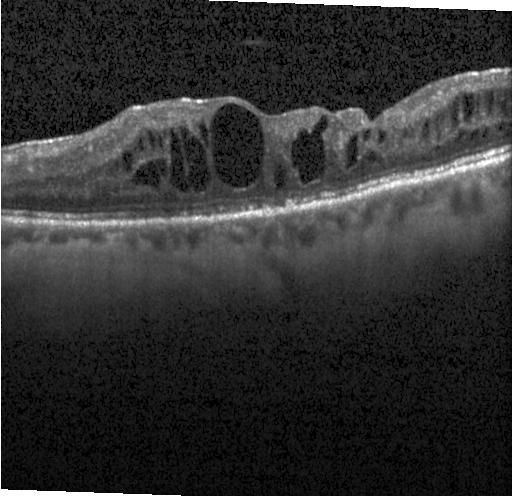 OCT B-scan; Heidelberg Spectralis OCT system; fovea-centered.
The scan shows DME.